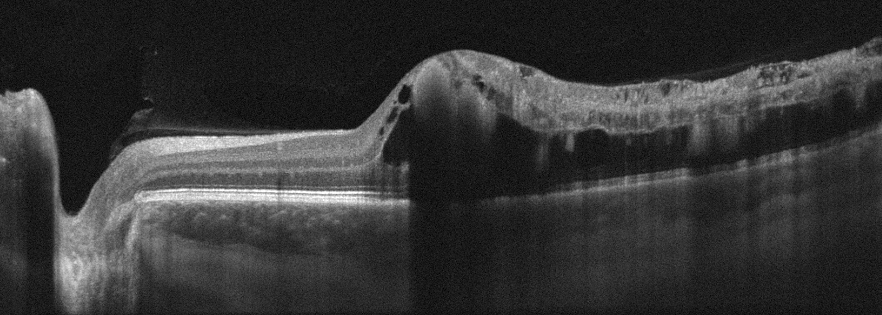
Optical coherence tomography scan; left eye; fovea-centered — Macular OCT: retinal vein occlusion (RVO).